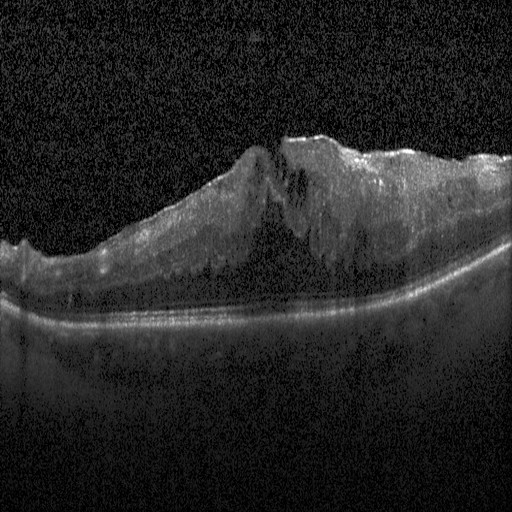 Spectral-domain optical coherence tomography. OCT B-scan
This B-scan demonstrates diabetic macular edema.